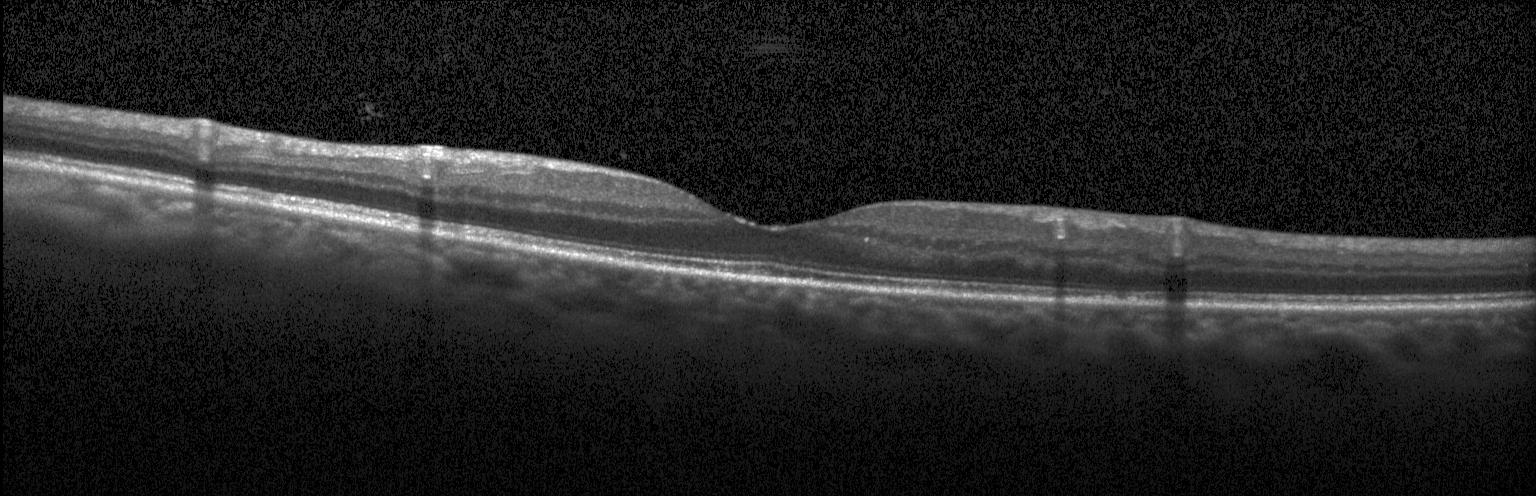

OCT B-scan.
This B-scan demonstrates neither choroidal neovascularization, diabetic macular edema, nor drusen.